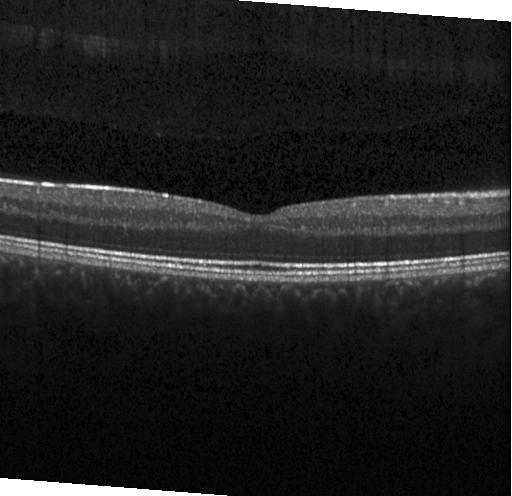
OCT line scan · centered on the fovea
Diagnosis: no choroidal neovascularization, diabetic macular edema, or drusen.